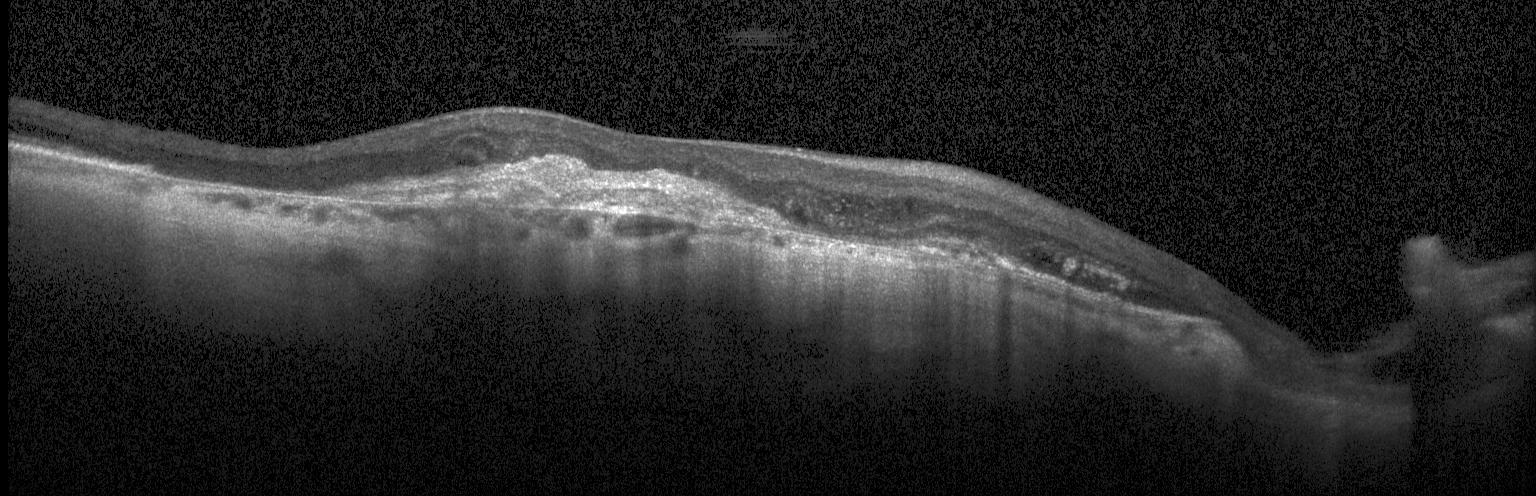

OCT line scan. Horizontal scan through the fovea.
OCT finding: a choroidal neovascular membrane.